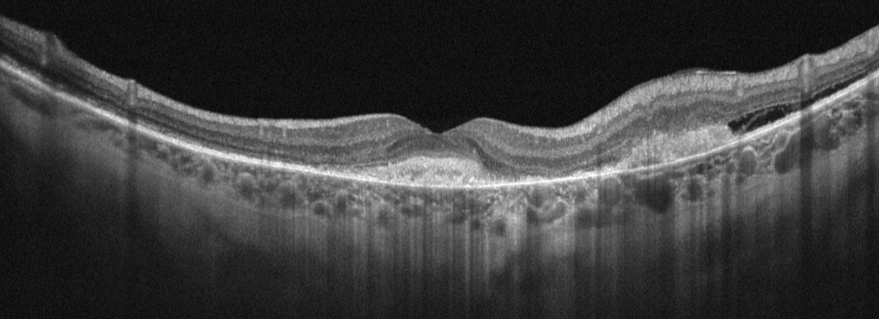
Retinal OCT B-scan
Impression: AMD.